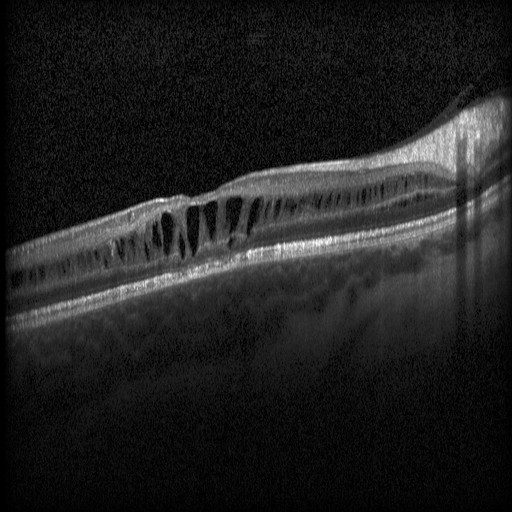 Spectral-domain OCT B-scan: diabetic macular edema.